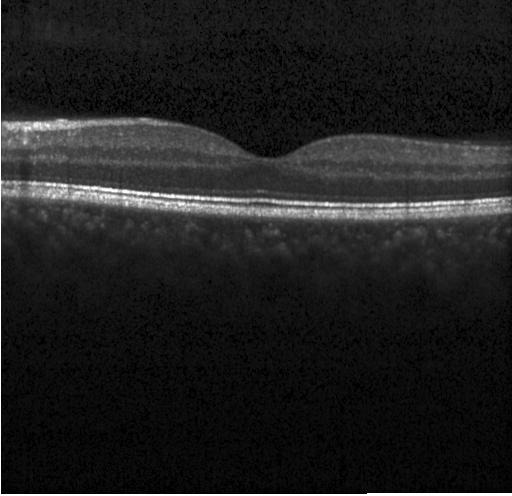

Finding: neither choroidal neovascularization, diabetic macular edema, nor drusen.